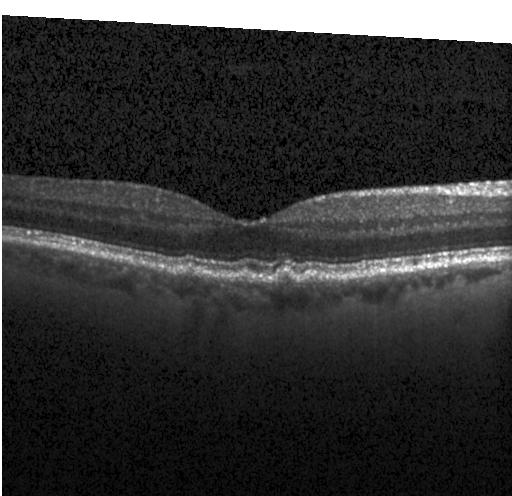 Fovea-centered. OCT line scan. Spectral-domain OCT. Acquired on a Heidelberg Spectralis. The scan shows sub-RPE drusenoid deposits.